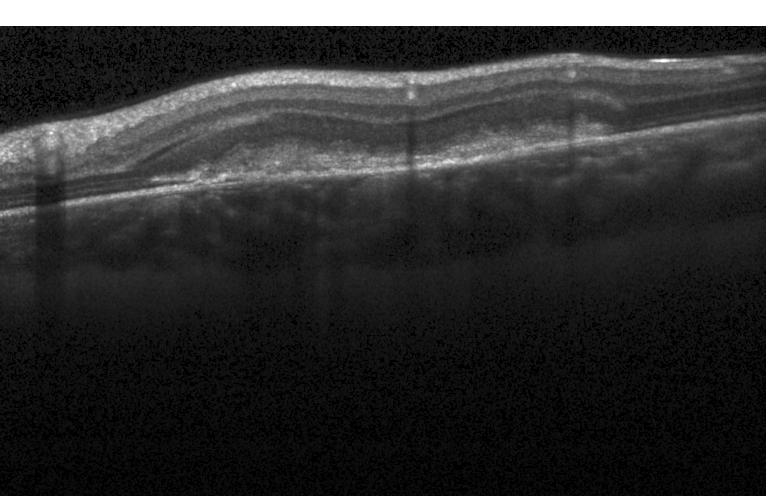
Macular OCT demonstrating a choroidal neovascular membrane.